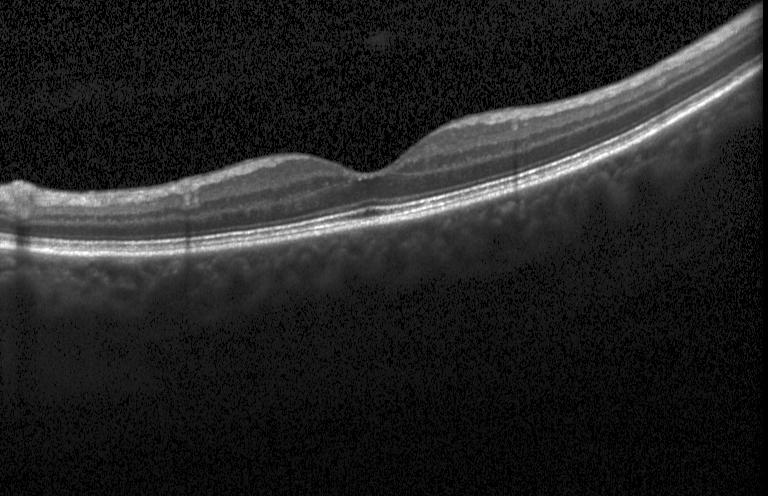
Optical coherence tomography scan. Spectral-domain optical coherence tomography. Instrument: Heidelberg Spectralis — Macular OCT: no evidence of choroidal neovascularization, diabetic macular edema, or drusen.